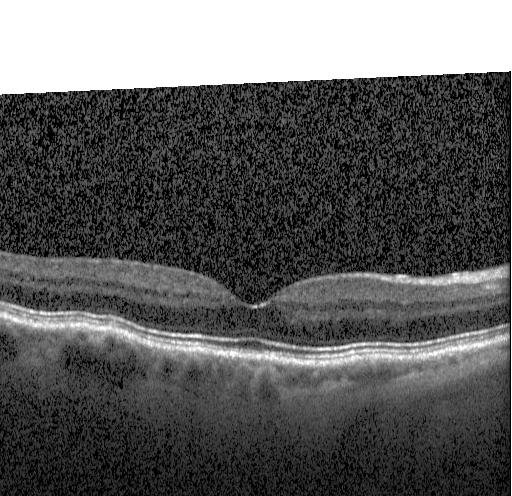
Spectral-domain OCT, Heidelberg Spectralis OCT system, horizontal scan through the fovea, OCT B-scan.
Finding: no evidence of choroidal neovascularization, diabetic macular edema, or drusen.